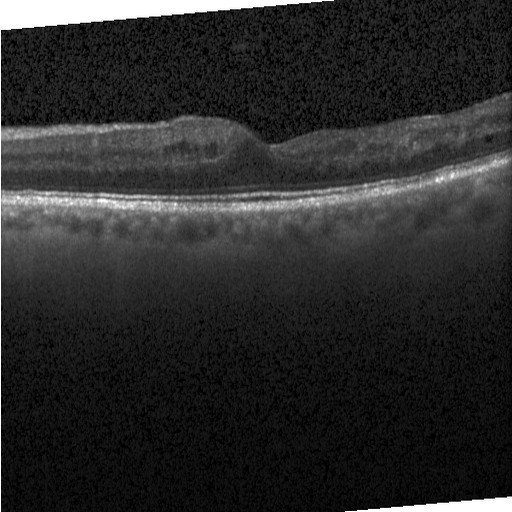 OCT finding: diabetic macular edema.